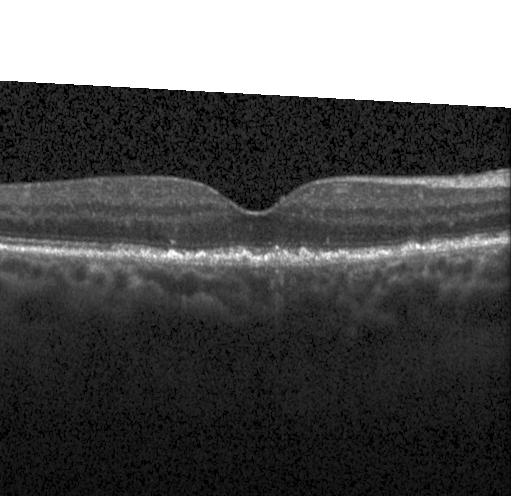

Macular scan; Heidelberg Spectralis; optical coherence tomography B-scan — Impression: drusen.